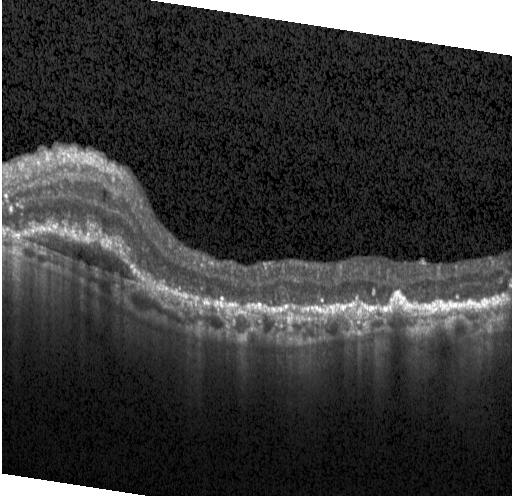
Optical coherence tomography B-scan, spectral-domain OCT, fovea-centered, acquired on a Heidelberg Spectralis.
Finding: choroidal neovascularization (CNV).